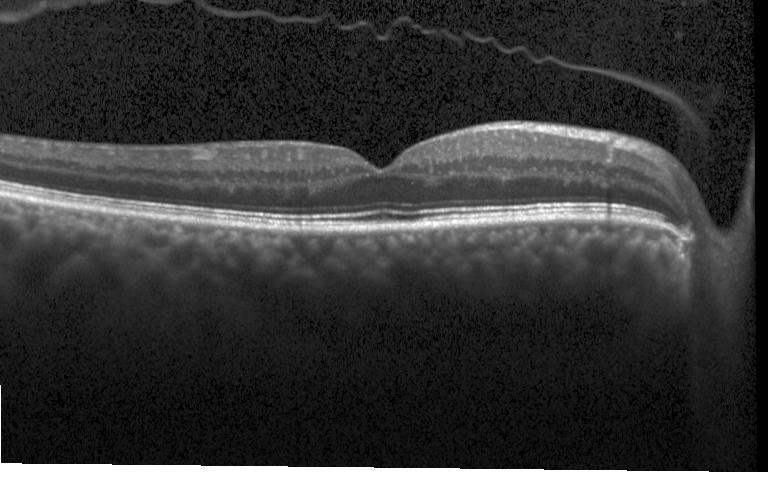

Optical coherence tomography scan; spectral-domain optical coherence tomography
Finding: no evidence of choroidal neovascularization, diabetic macular edema, or drusen.